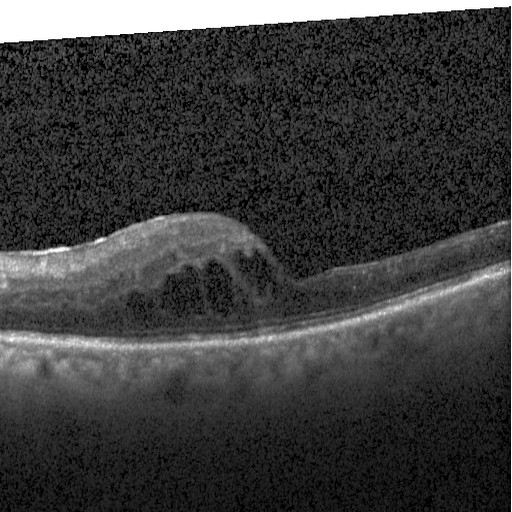
OCT B-scan — Dx: diabetic macular edema.